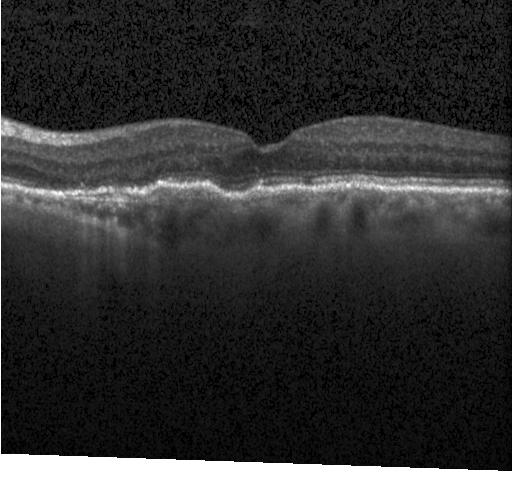
Impression: choroidal neovascularization.